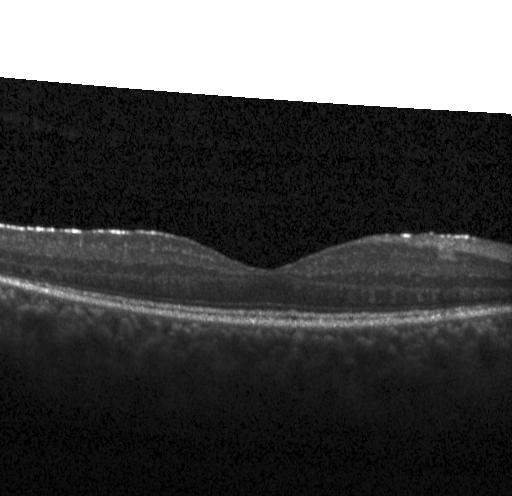

The scan shows no choroidal neovascularization, no diabetic macular edema, and no drusen.